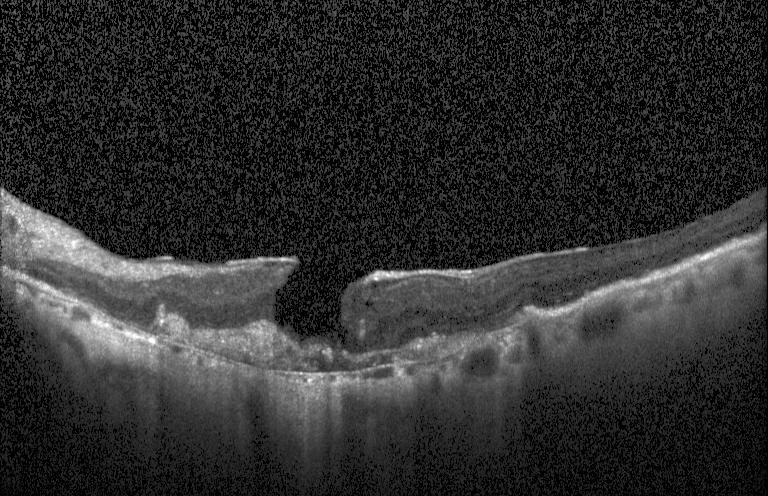
Optical coherence tomography scan, centered on the fovea
This B-scan demonstrates choroidal neovascularization (CNV).